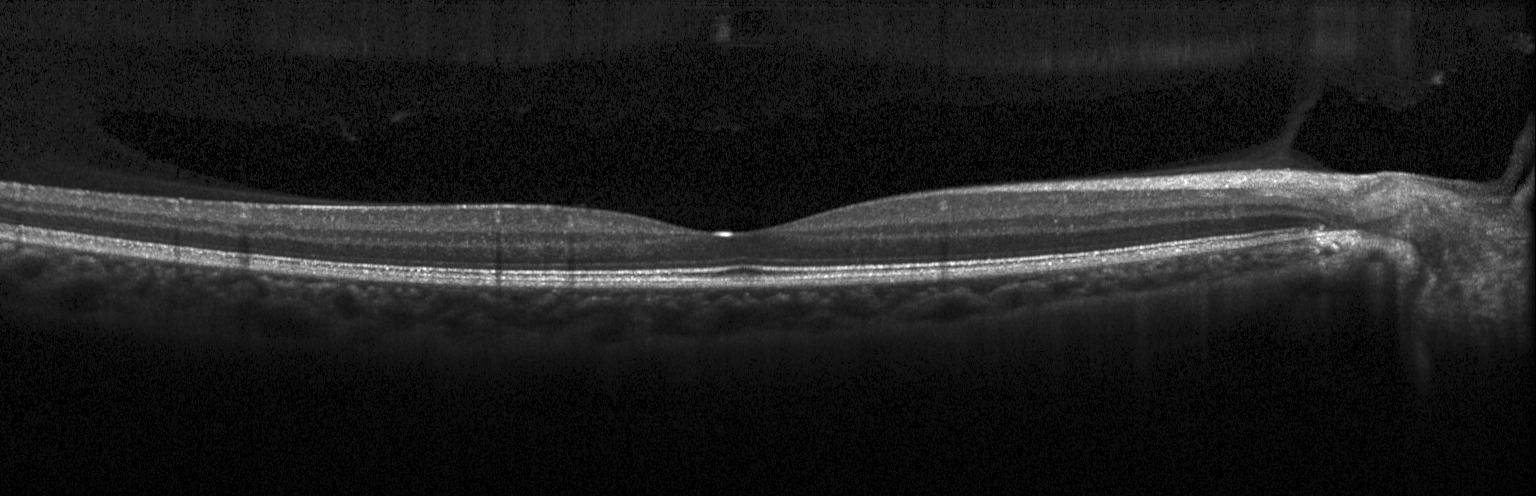 Spectral-domain OCT · OCT line scan · through the macula.
Assessment: neither choroidal neovascularization, diabetic macular edema, nor drusen.